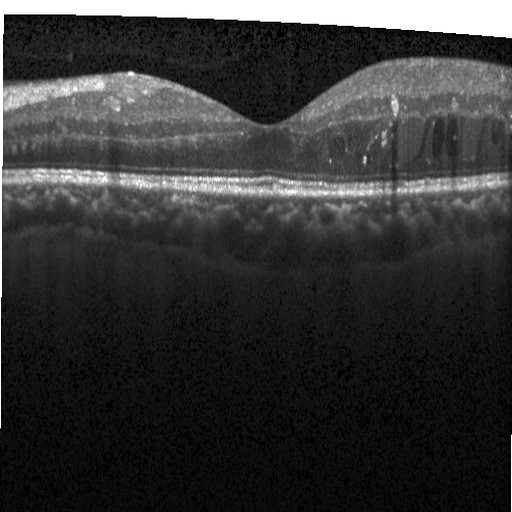 Finding: DME.